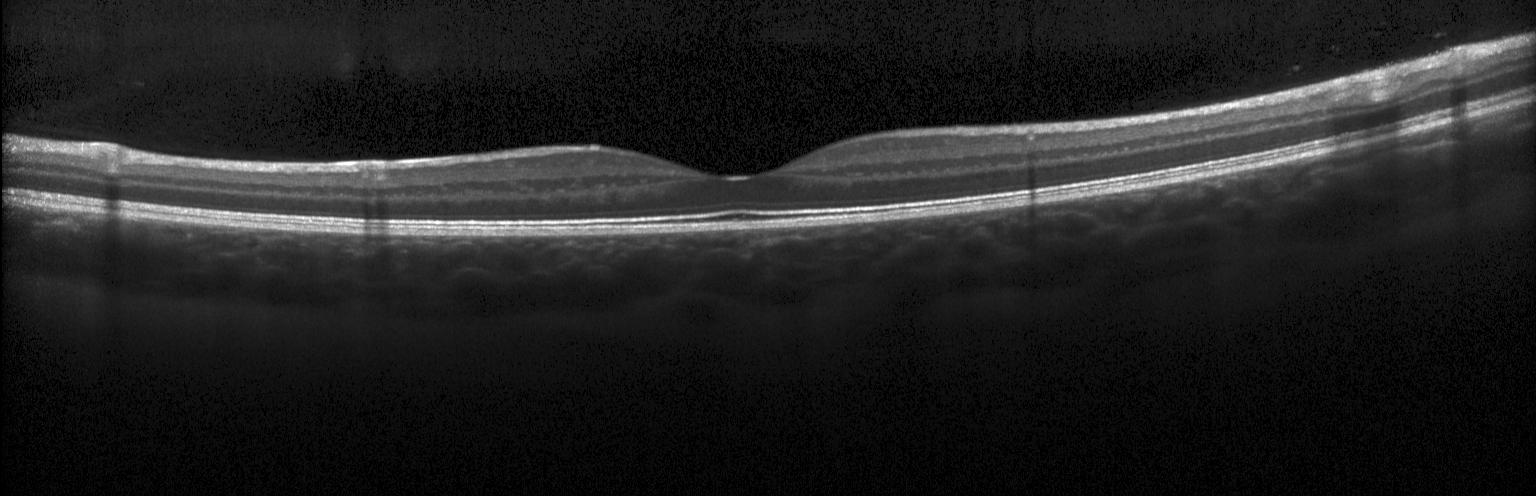
Horizontal scan through the fovea. Retinal OCT cross-section. This B-scan demonstrates no choroidal neovascularization, no diabetic macular edema, and no drusen.